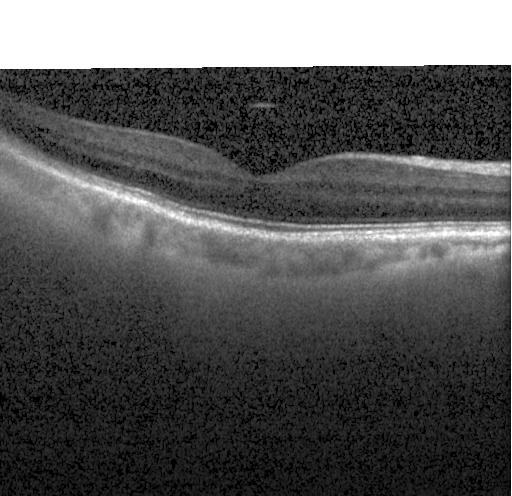

Spectral-domain optical coherence tomography · centered on the fovea · OCT line scan — Diagnosis: no choroidal neovascularization, diabetic macular edema, or drusen.